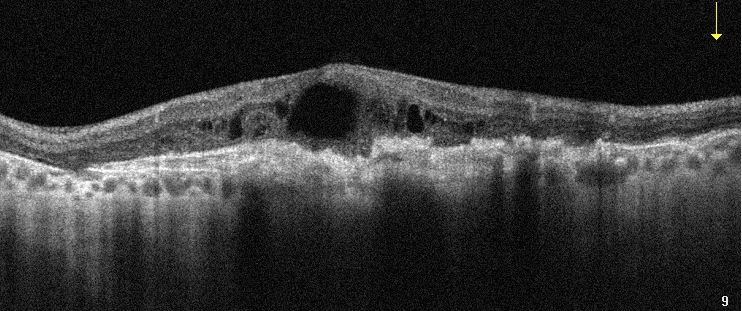

Diagnosis: age-related macular degeneration.